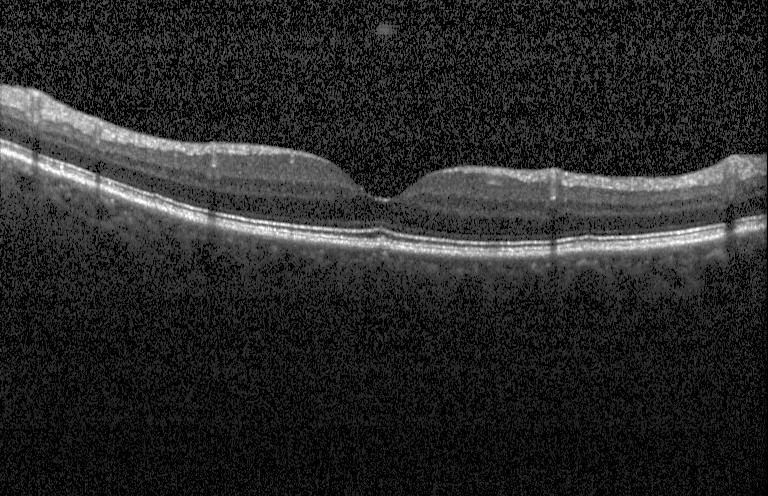
Diagnosis: neither choroidal neovascularization, diabetic macular edema, nor drusen.